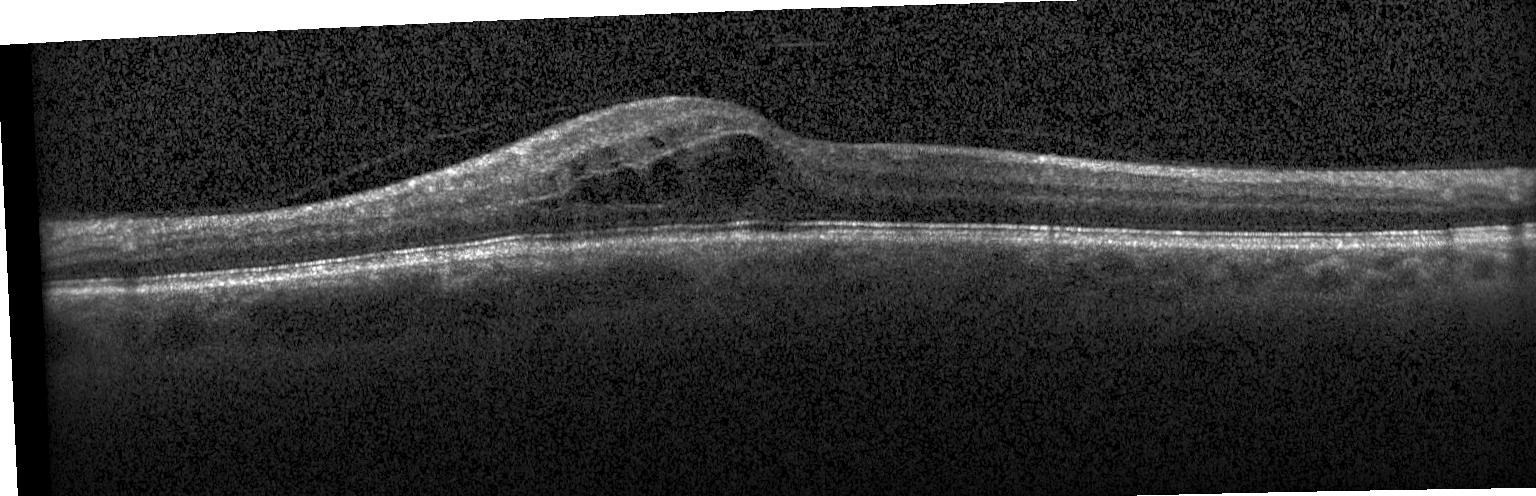

This B-scan demonstrates diabetic macular edema.